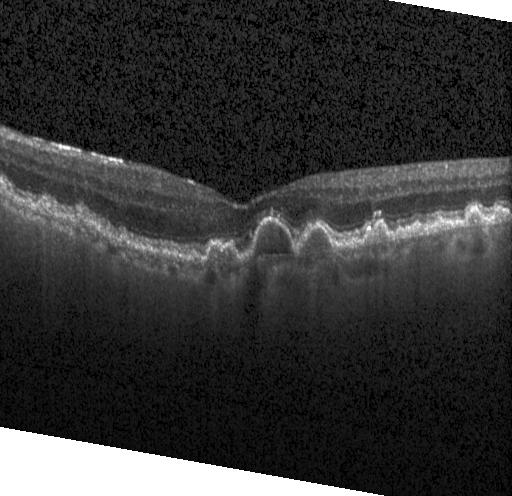
Finding: drusen.